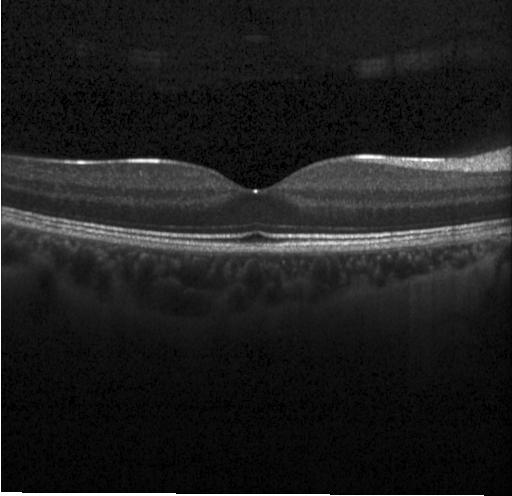 Centered on the fovea. Optical coherence tomography scan. SD-OCT. Heidelberg Spectralis.
No choroidal neovascularization, diabetic macular edema, or drusen.